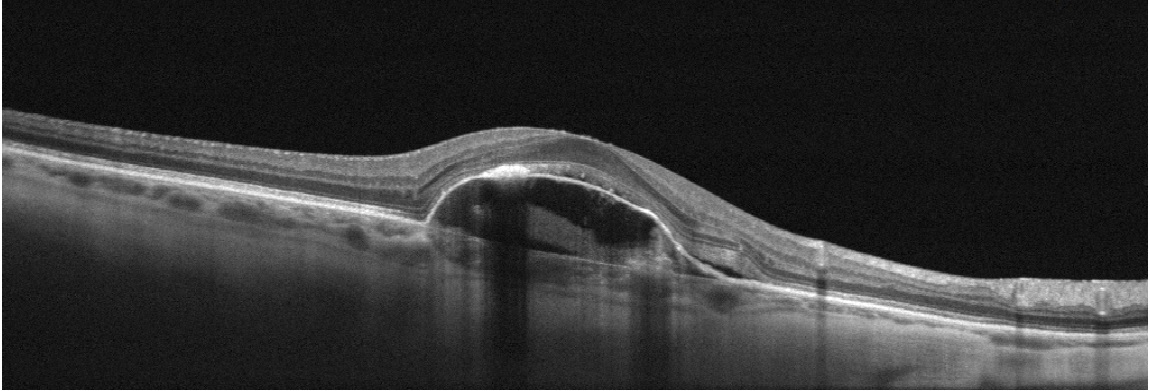

OCT line scan — Impression: age-related macular degeneration (AMD).